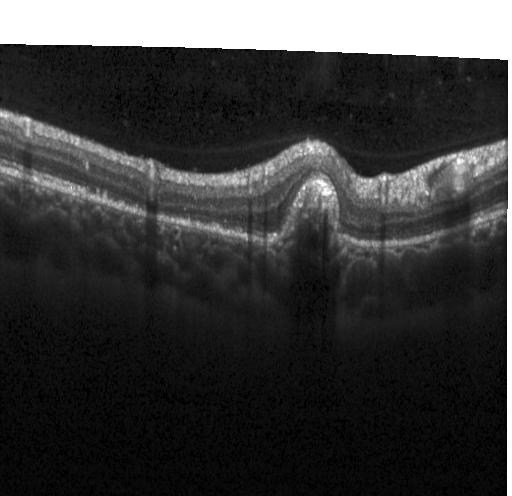
Optical coherence tomography B-scan. SD-OCT — Impression: a choroidal neovascular membrane.